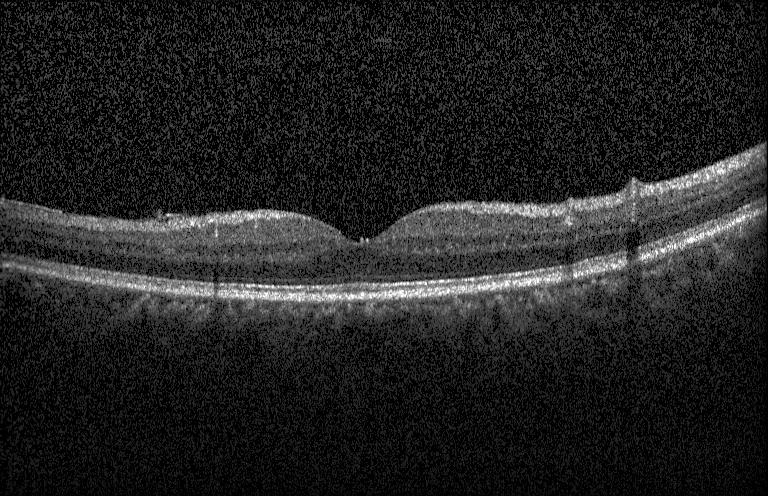

Centered on the fovea · retinal OCT cross-section
Diagnosis: no CNV, no DME, and no drusen.